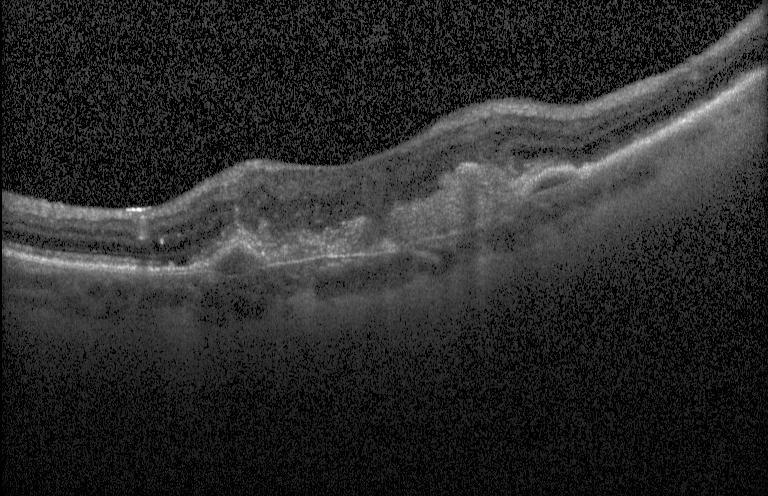
Acquired on a Heidelberg Spectralis. Retinal OCT cross-section. Fovea-centered
The scan shows a choroidal neovascular membrane.